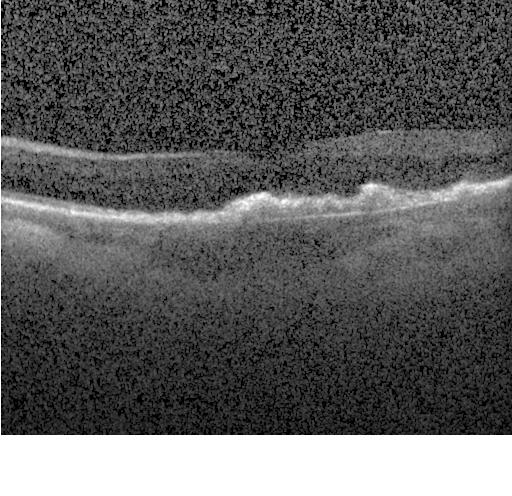

Finding: choroidal neovascularization.